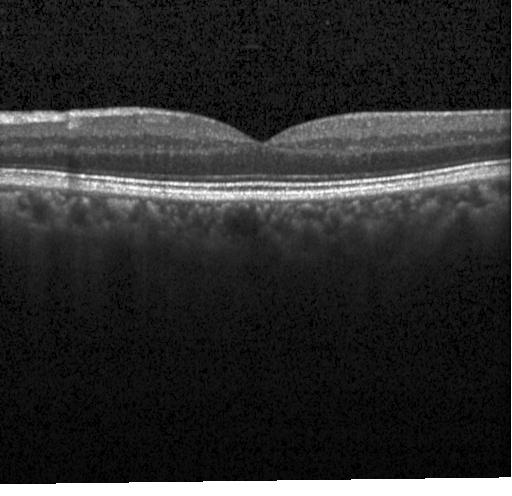 OCT line scan, fovea-centered, instrument: Heidelberg Spectralis, SD-OCT. Finding: no evidence of choroidal neovascularization, diabetic macular edema, or drusen.